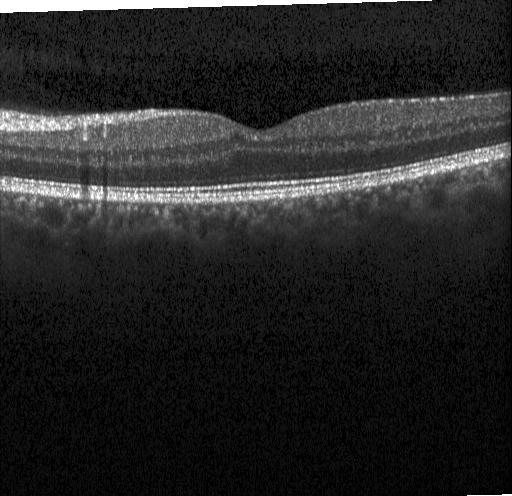

Macular scan, Heidelberg Spectralis, optical coherence tomography B-scan. Finding: no CNV, DME, or drusen.